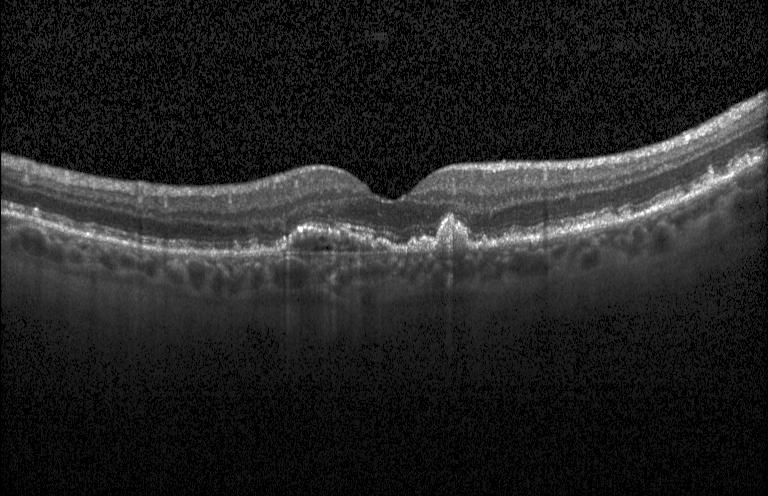
OCT scan showing choroidal neovascularization (CNV).